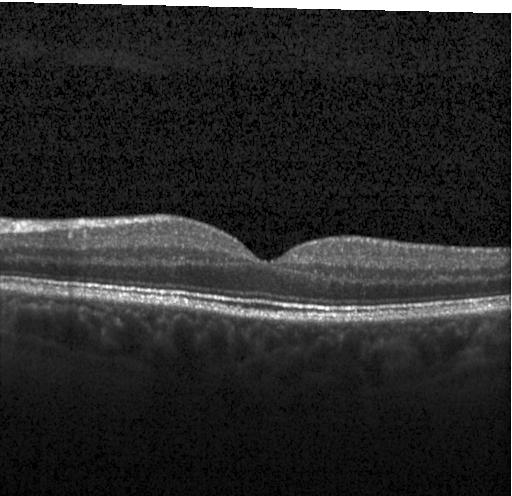 Impression: no choroidal neovascularization, no diabetic macular edema, and no drusen.